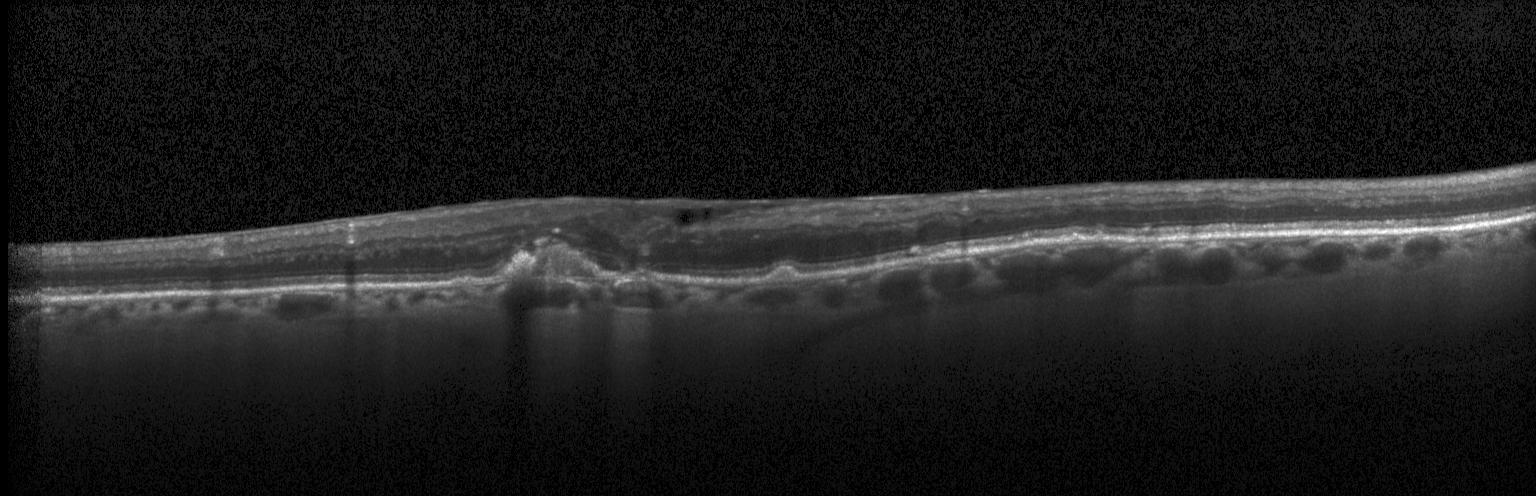

Acquired on a Heidelberg Spectralis. OCT B-scan — Impression: a choroidal neovascular membrane.